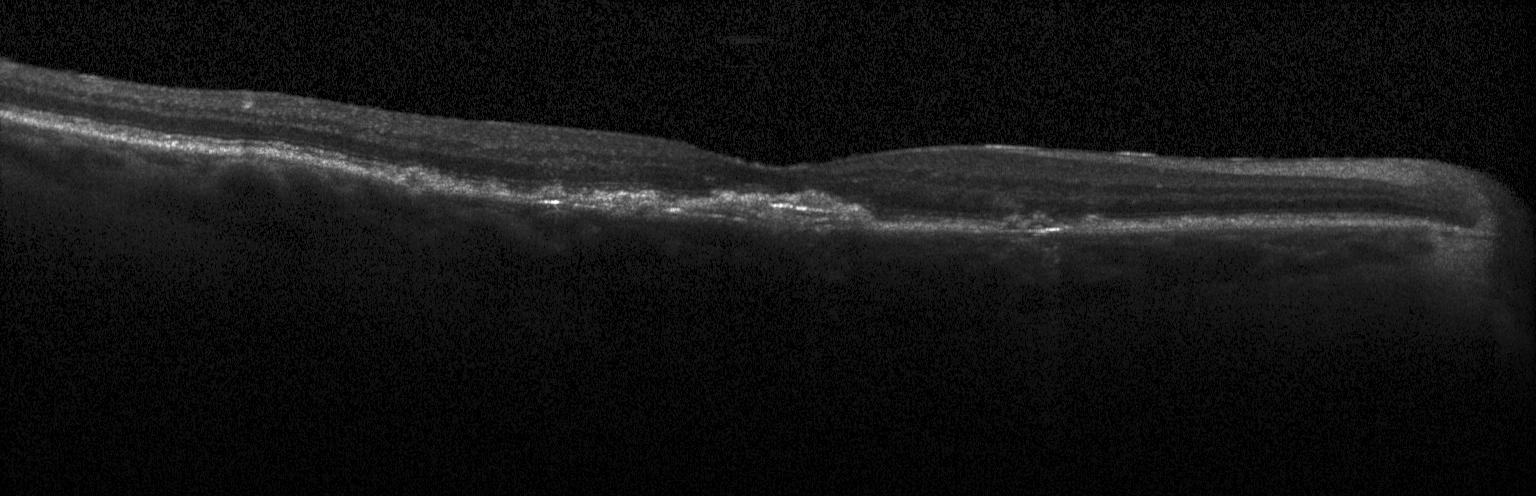

Diagnosis: CNV.